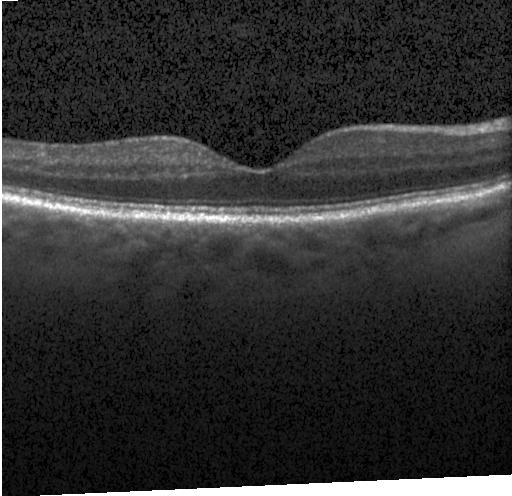

Retinal OCT B-scan. Finding: no CNV, DME, or drusen.